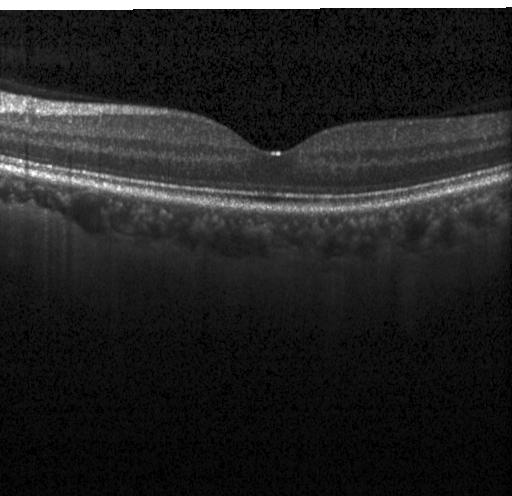
OCT scan showing neither choroidal neovascularization, diabetic macular edema, nor drusen.